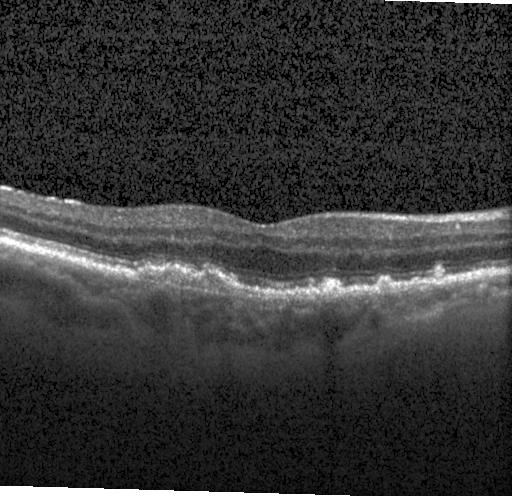

Heidelberg Spectralis OCT system, SD-OCT, centered on the fovea, optical coherence tomography B-scan
Assessment: a choroidal neovascular membrane.